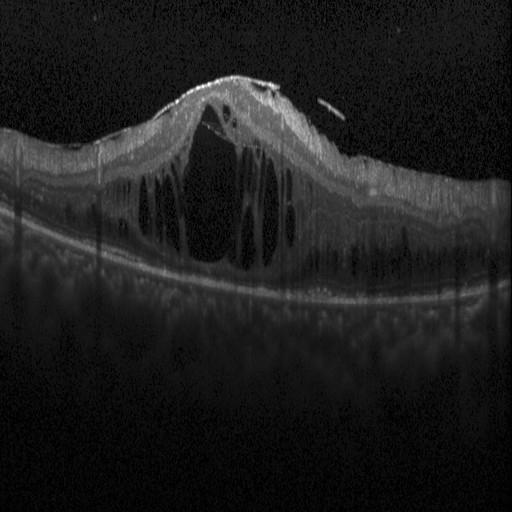
Retinal OCT cross-section
Diagnosis: diabetic macular edema.